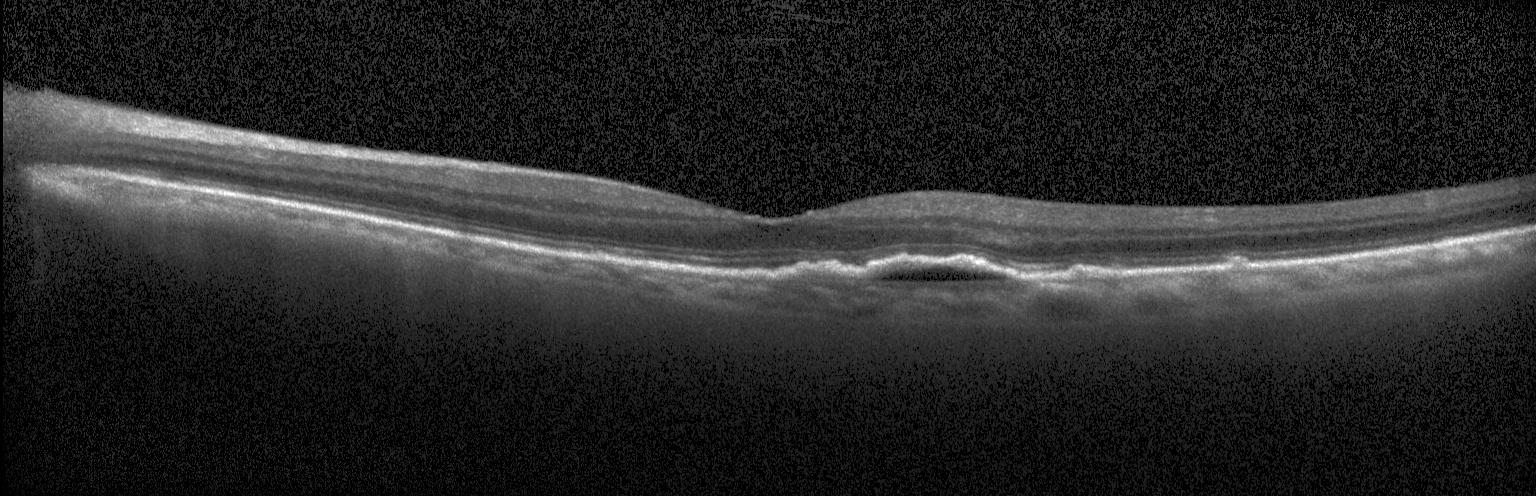

OCT B-scan showing a choroidal neovascular membrane.